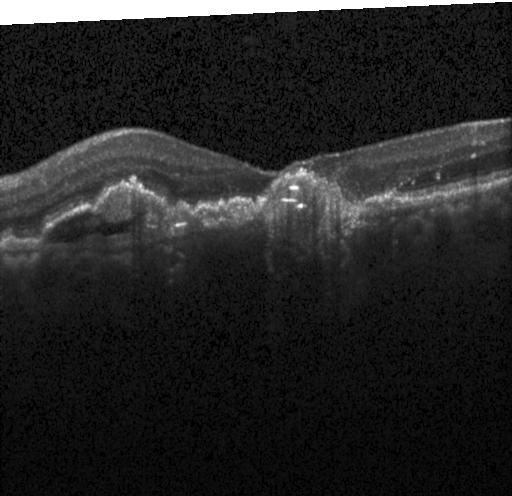 Retinal OCT B-scan; Heidelberg Spectralis OCT system.
OCT finding: a choroidal neovascular membrane.